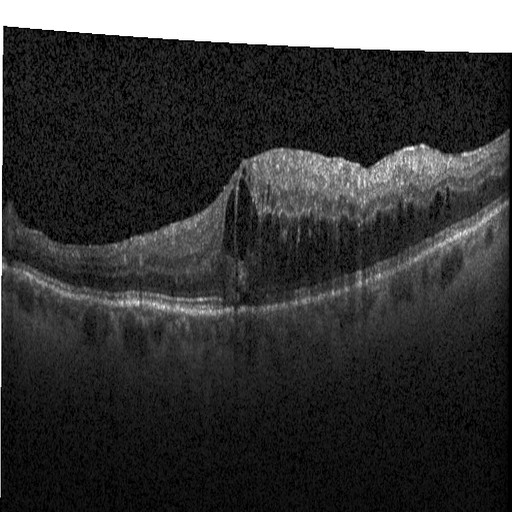

Assessment: DME.